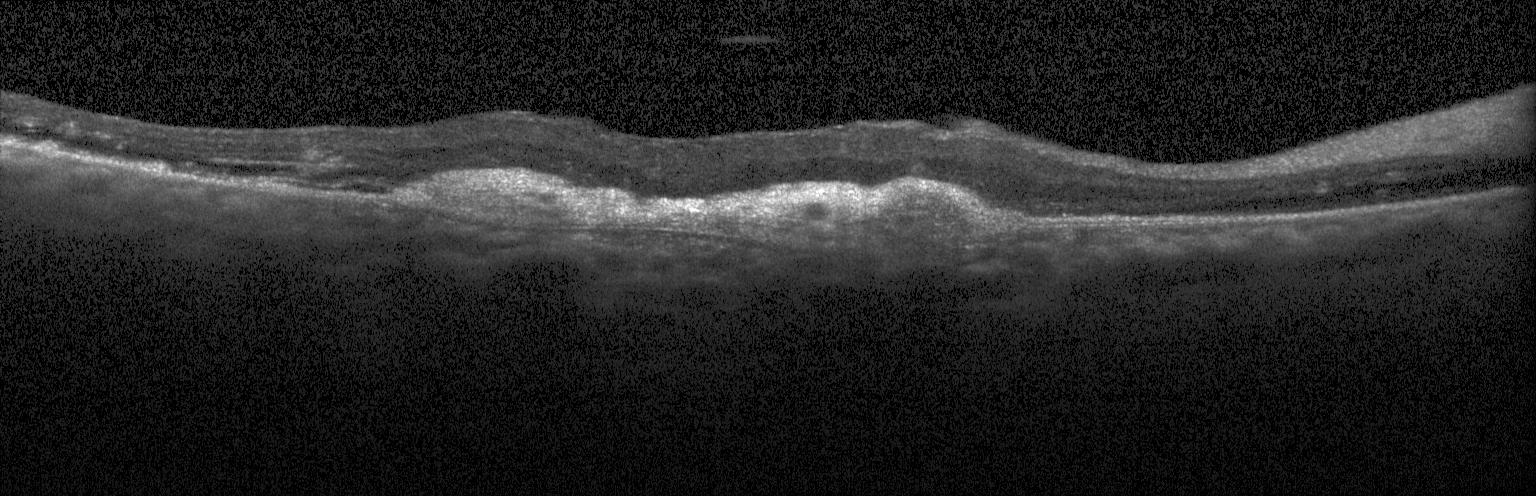 Diagnosis: a choroidal neovascular membrane.